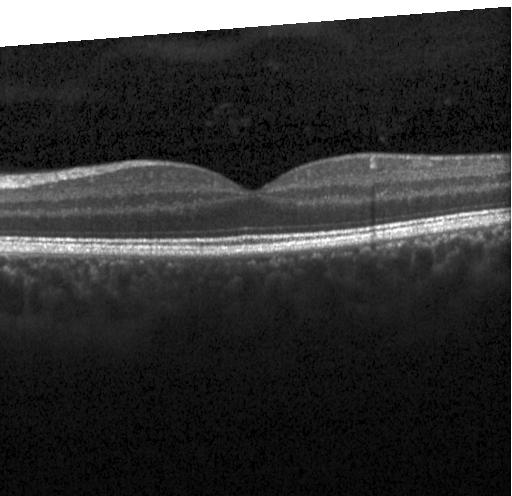

SD-OCT · centered on the fovea · OCT B-scan · Heidelberg Spectralis OCT system
Finding: no choroidal neovascularization, diabetic macular edema, or drusen.